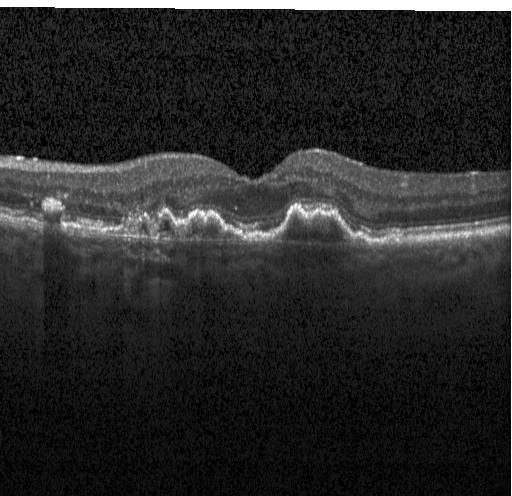
Assessment: a choroidal neovascular membrane.